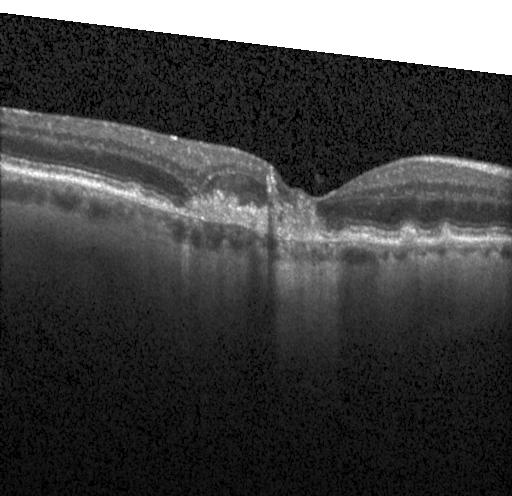 Diagnosis: a choroidal neovascular membrane.